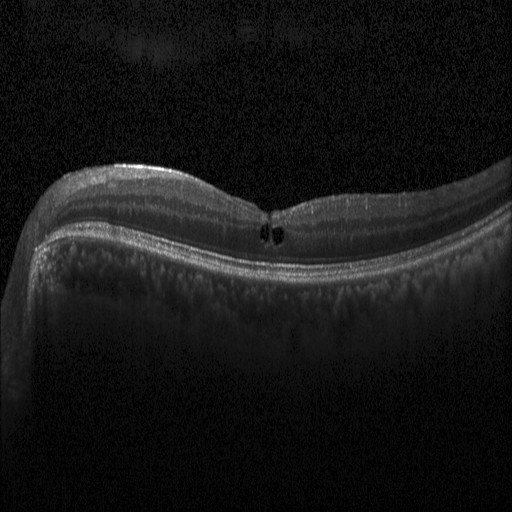
Impression: DME.